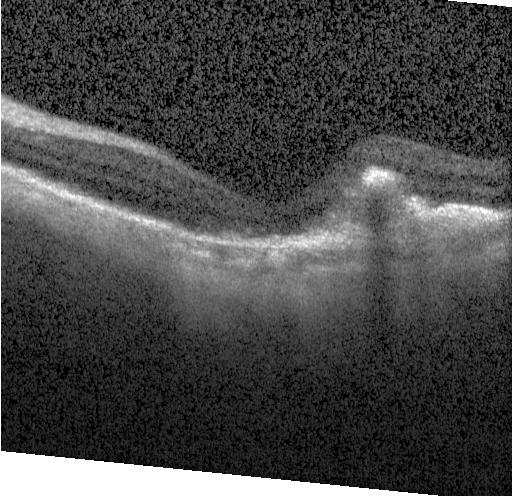
Retinal OCT B-scan. Fovea-centered. Instrument: Heidelberg Spectralis. Assessment: a choroidal neovascular membrane.